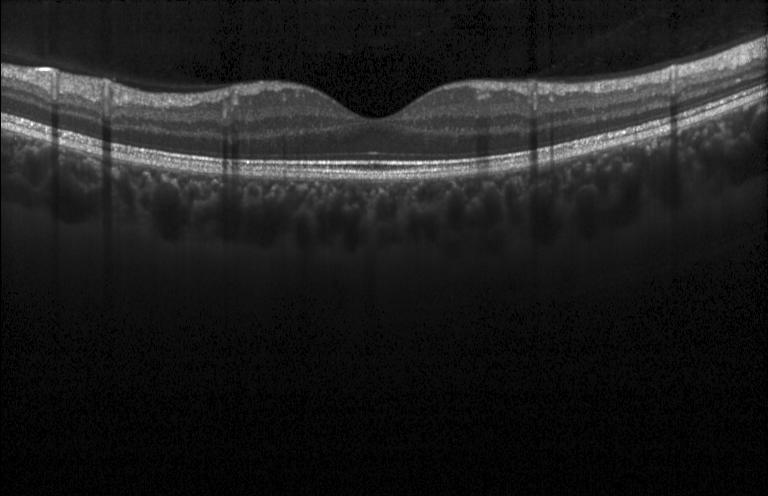
Macular OCT: neither choroidal neovascularization, diabetic macular edema, nor drusen.